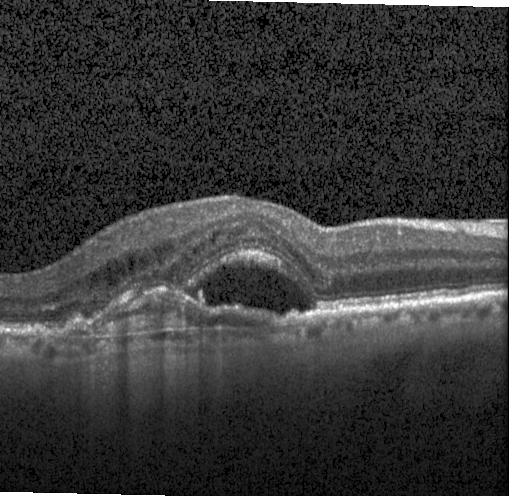 Diagnosis: choroidal neovascularization.